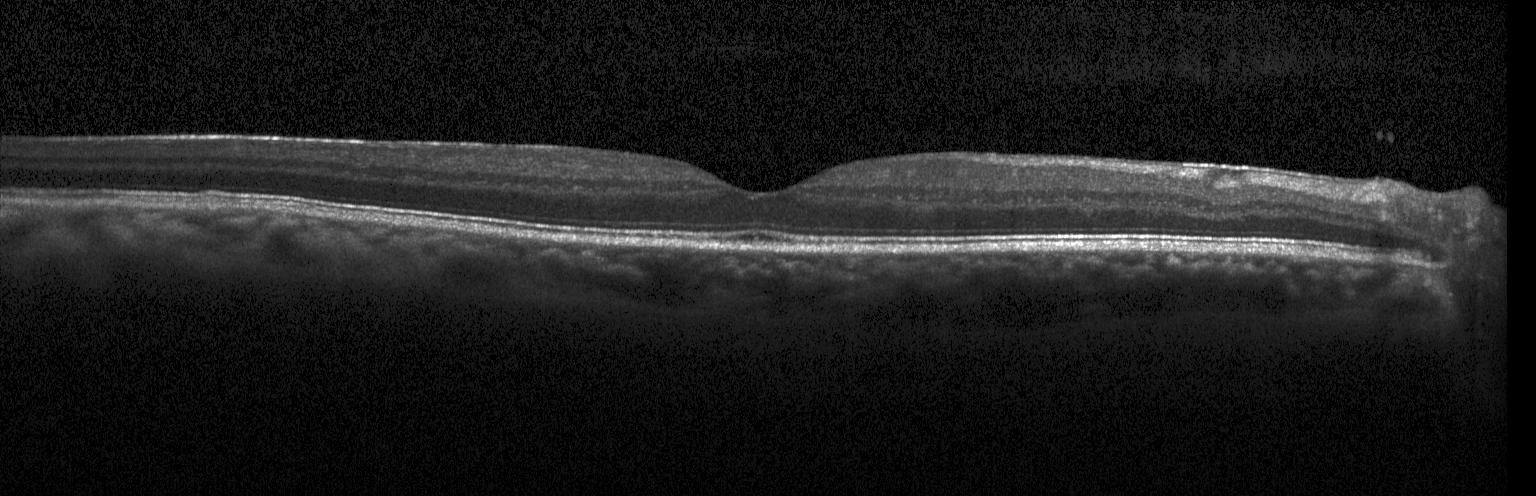 Finding: neither choroidal neovascularization, diabetic macular edema, nor drusen.